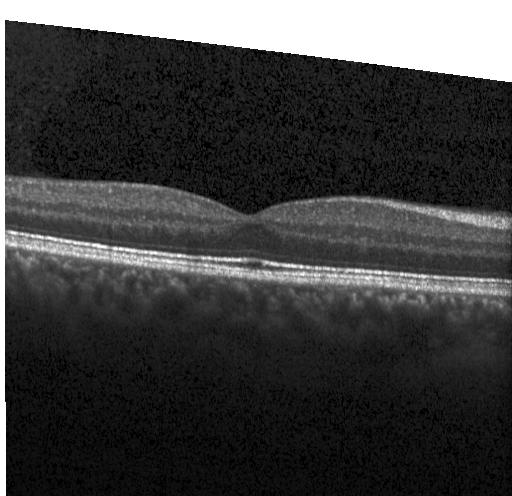 Spectral-domain optical coherence tomography; retinal OCT cross-section. Diagnosis: neither choroidal neovascularization, diabetic macular edema, nor drusen.